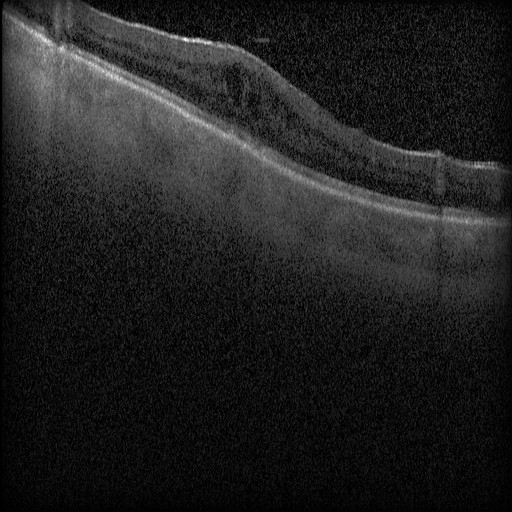
Diabetic macular edema (DME).